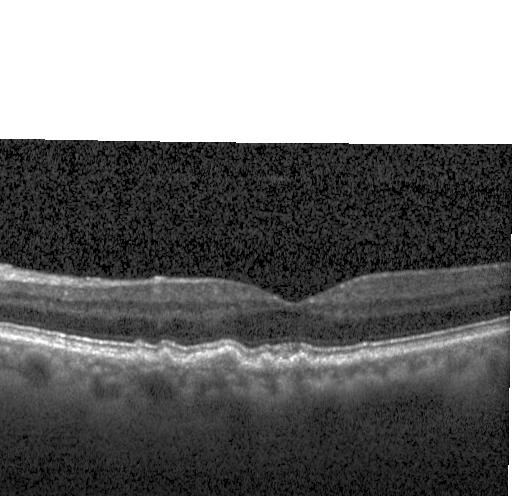

Macular scan. Retinal OCT B-scan. Acquired on a Heidelberg Spectralis. Spectral-domain OCT — Impression: sub-RPE drusenoid deposits.